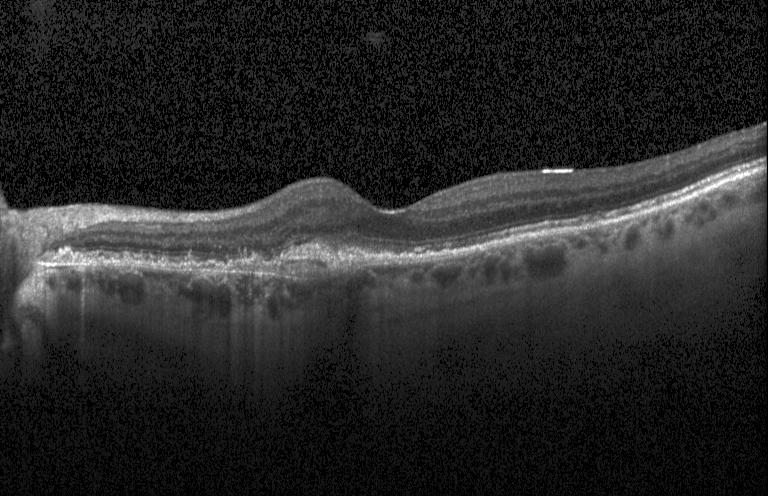
Retinal OCT B-scan. SD-OCT. Instrument: Heidelberg Spectralis. Through the macula — A choroidal neovascular membrane.